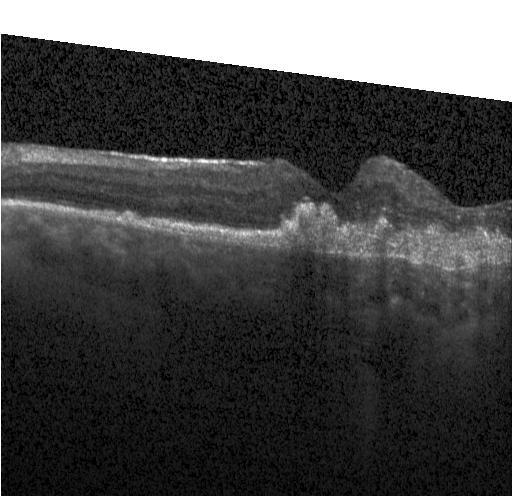
Optical coherence tomography B-scan — This B-scan demonstrates choroidal neovascularization (CNV).